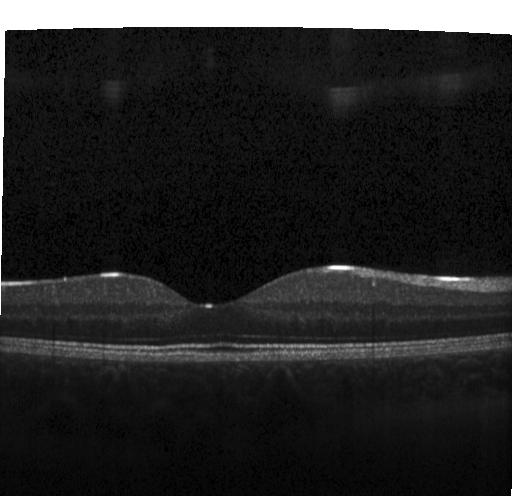

Macular scan, Heidelberg Spectralis, OCT B-scan, SD-OCT — The scan shows neither CNV, DME, nor drusen.